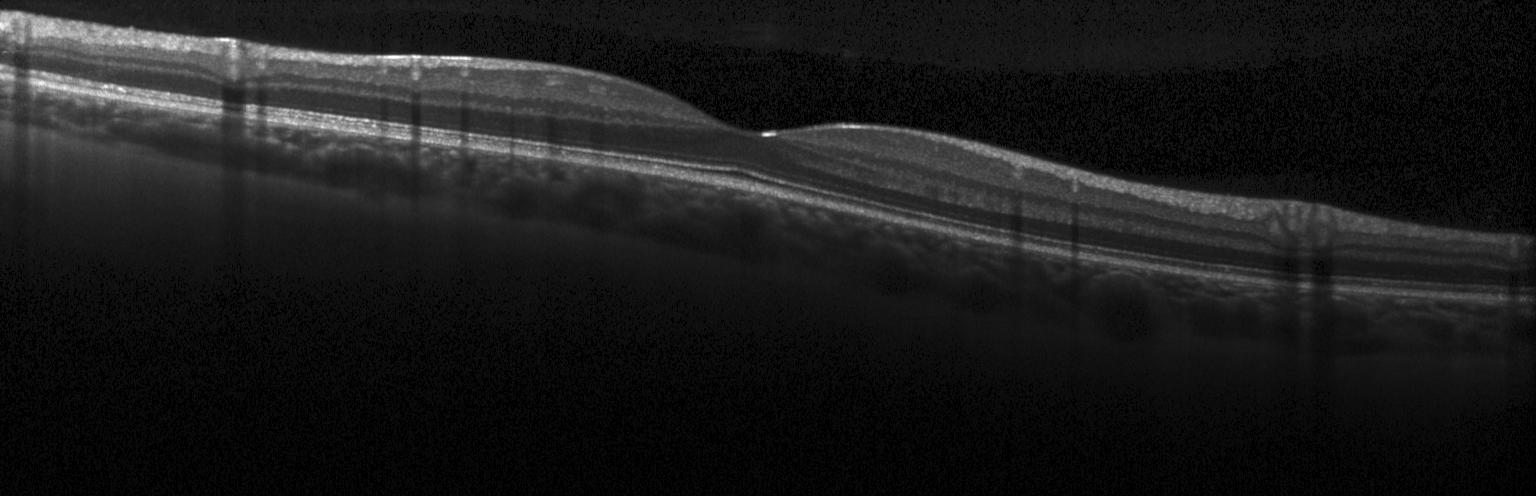

Finding: no choroidal neovascularization, no diabetic macular edema, and no drusen.